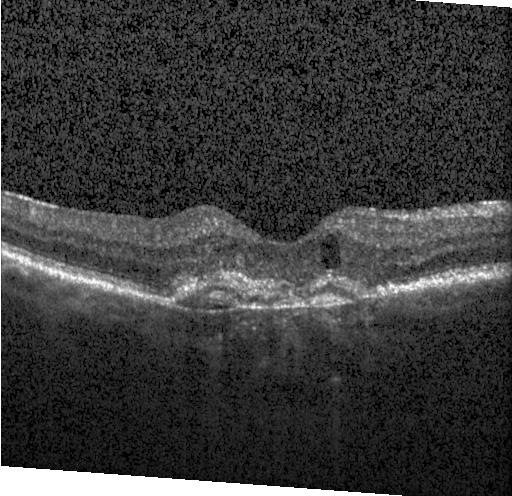 Retinal OCT cross-section. Spectral-domain OCT
Finding: a choroidal neovascular membrane.